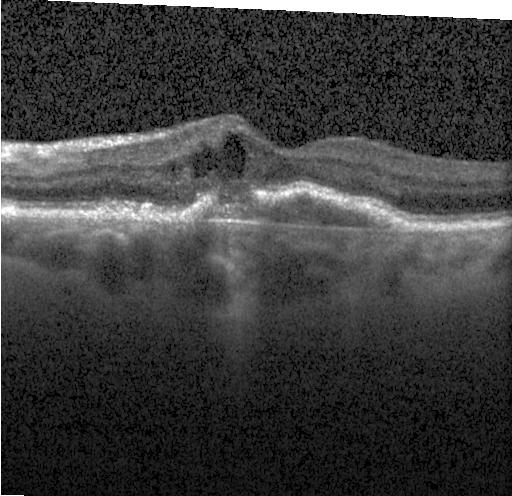
SD-OCT, OCT B-scan, macular scan — Dx: a choroidal neovascular membrane.